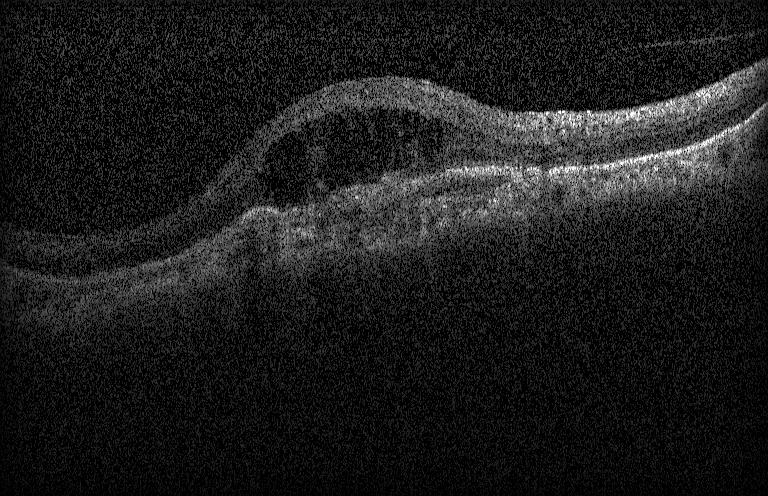

Optical coherence tomography scan.
Diagnosis: a choroidal neovascular membrane.